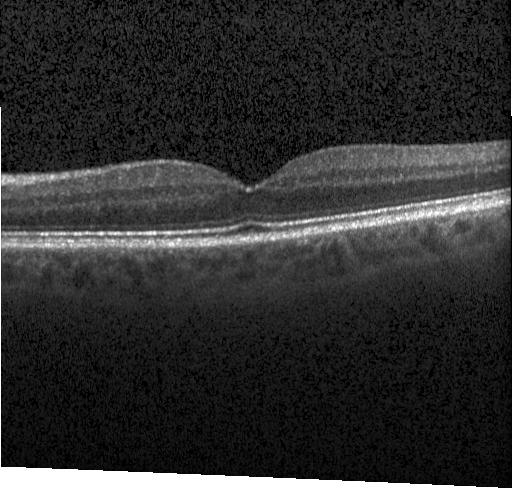
Optical coherence tomography B-scan. Heidelberg Spectralis OCT system
OCT finding: no choroidal neovascularization, no diabetic macular edema, and no drusen.